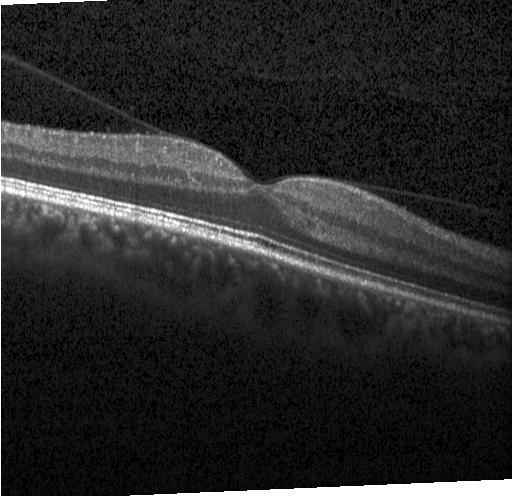

Assessment: neither CNV, DME, nor drusen.